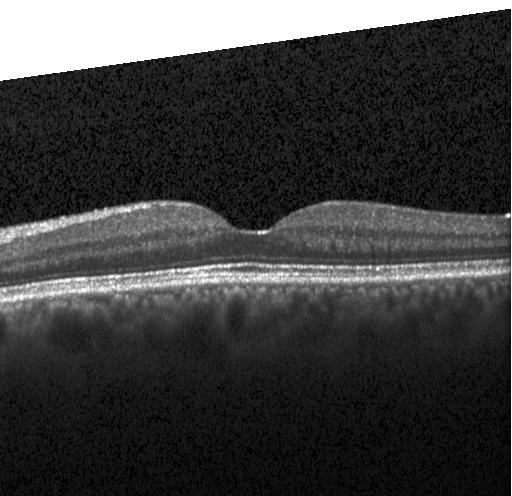

Dx: no evidence of choroidal neovascularization, diabetic macular edema, or drusen.